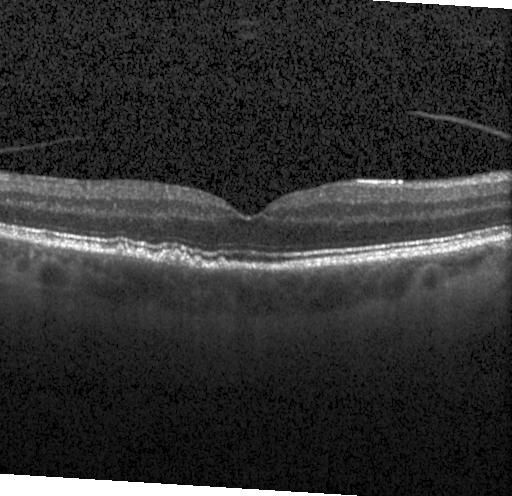
Finding: sub-RPE drusenoid deposits.